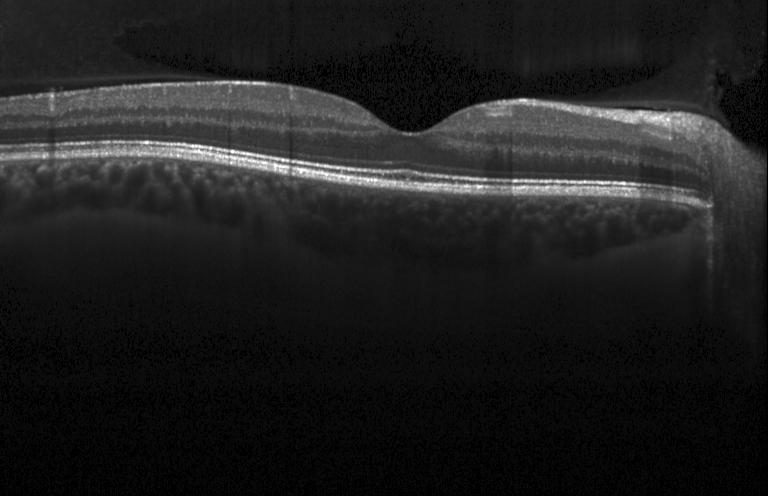 Acquired on a Heidelberg Spectralis. OCT line scan. SD-OCT.
The scan shows neither choroidal neovascularization, diabetic macular edema, nor drusen.